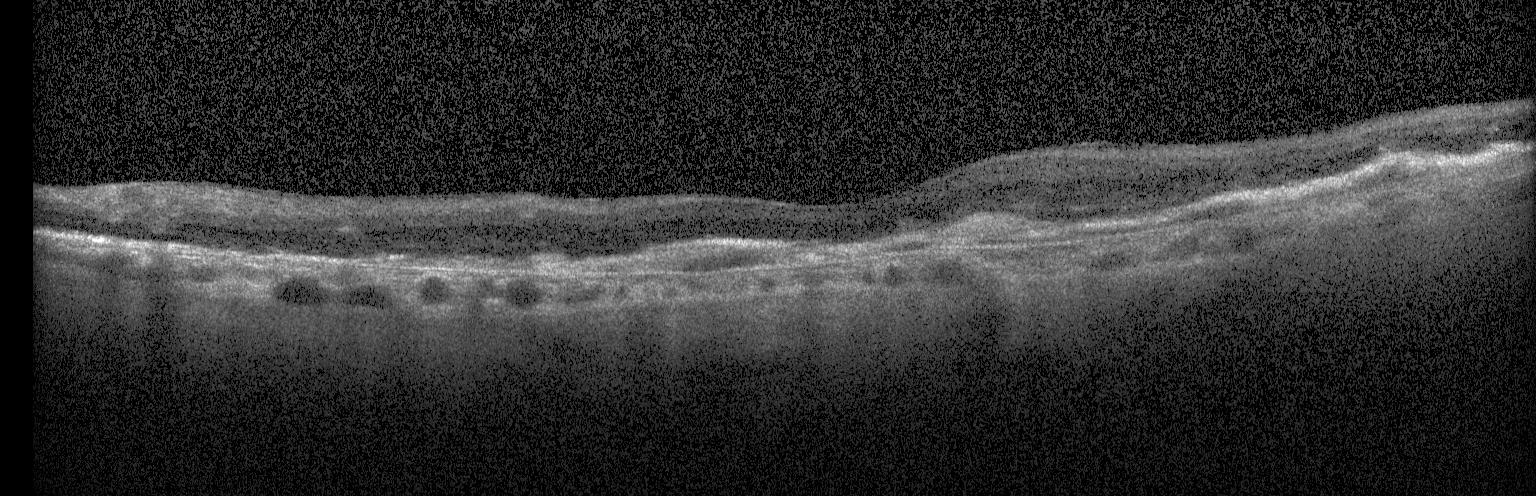
Heidelberg Spectralis OCT system · spectral-domain optical coherence tomography · optical coherence tomography B-scan · through the macula — Choroidal neovascularization.